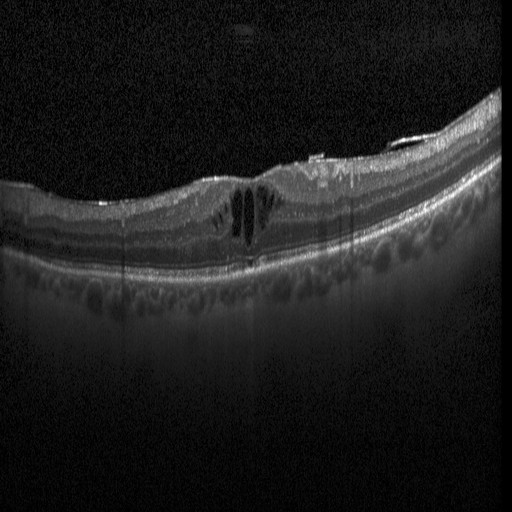

Macular OCT demonstrating diabetic macular edema (DME).